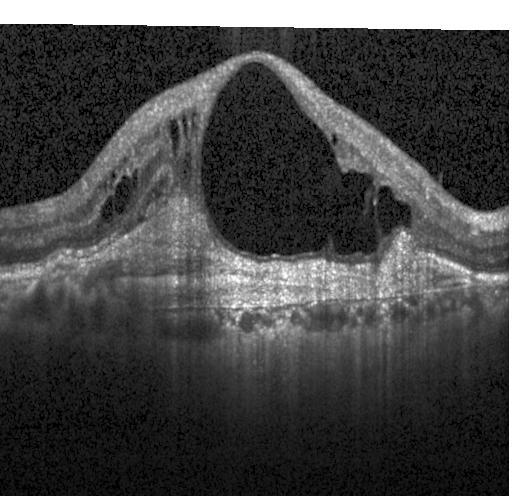 OCT line scan.
Impression: CNV.